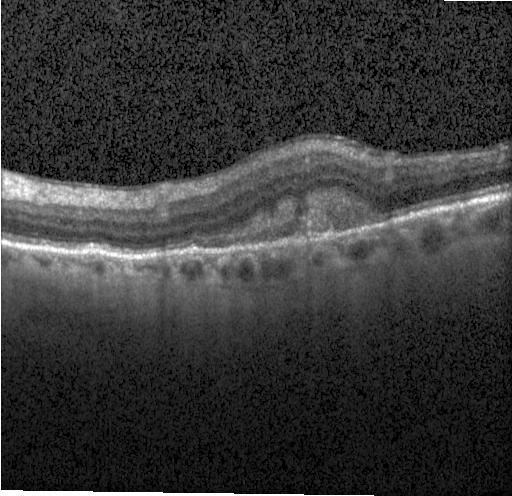

Dx: choroidal neovascularization (CNV).